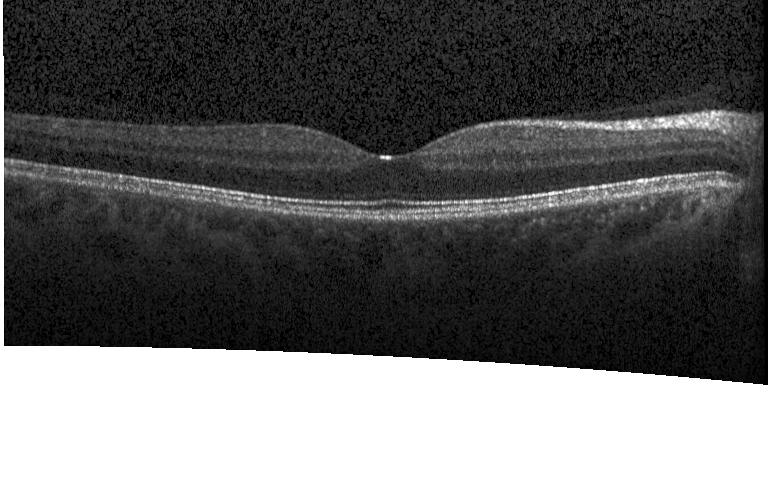 Optical coherence tomography B-scan. Horizontal scan through the fovea. Acquired on a Heidelberg Spectralis. SD-OCT — The scan shows neither choroidal neovascularization, diabetic macular edema, nor drusen.